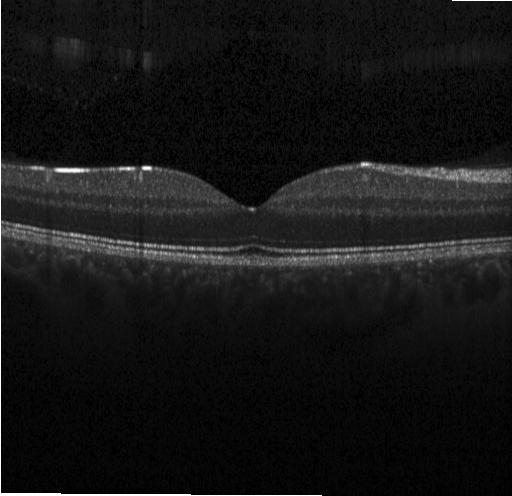

Assessment: neither CNV, DME, nor drusen.